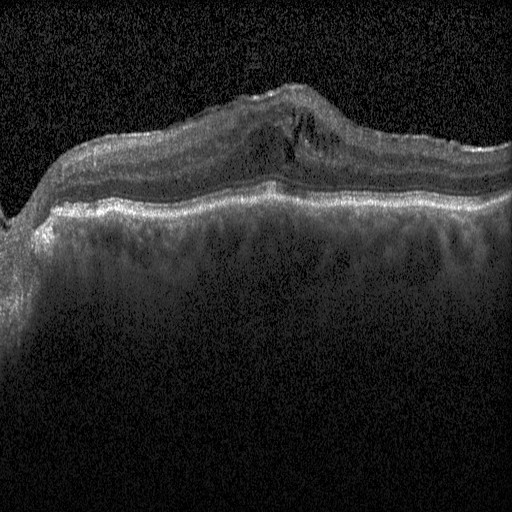
Retinal OCT B-scan. Finding: diabetic macular edema (DME).